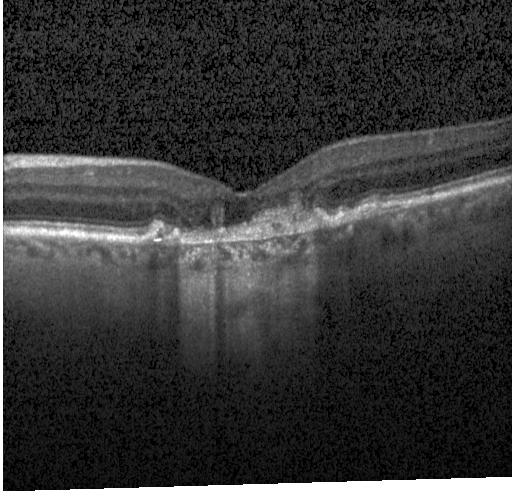
Through the macula; OCT line scan. The scan shows CNV.